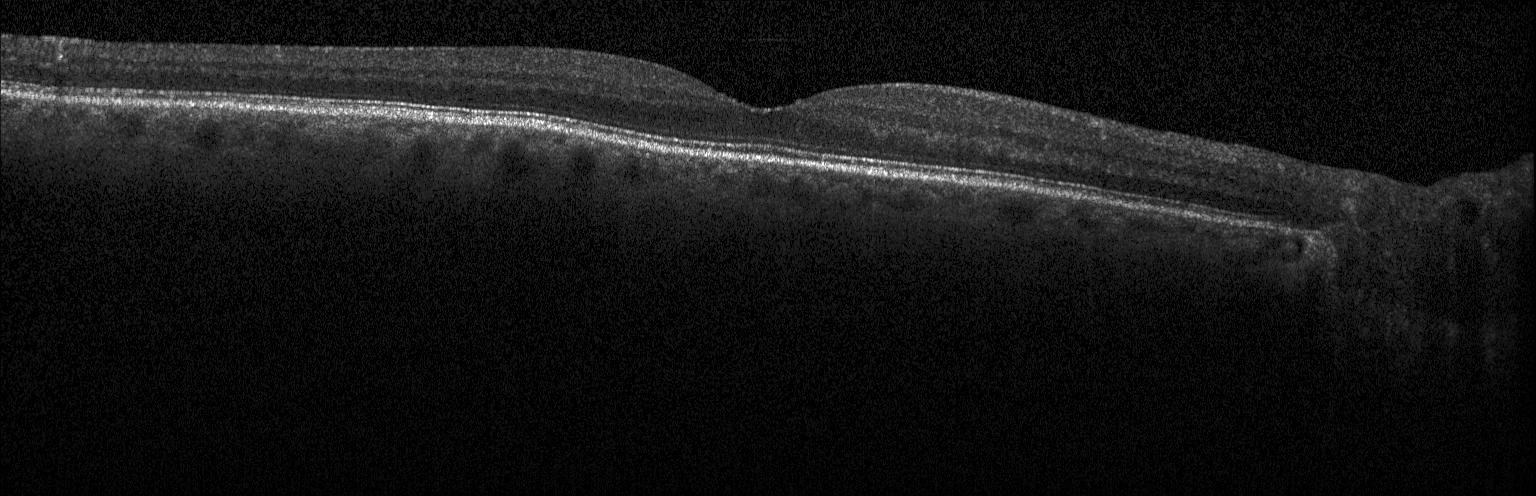
OCT line scan; fovea-centered — The scan shows no choroidal neovascularization, no diabetic macular edema, and no drusen.